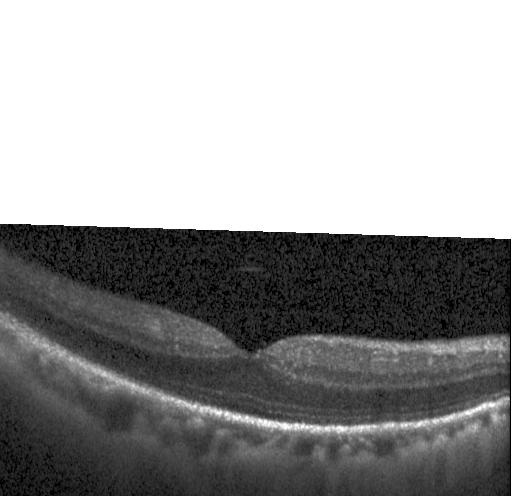

Centered on the fovea. Optical coherence tomography scan. SD-OCT. This B-scan demonstrates no choroidal neovascularization, no diabetic macular edema, and no drusen.